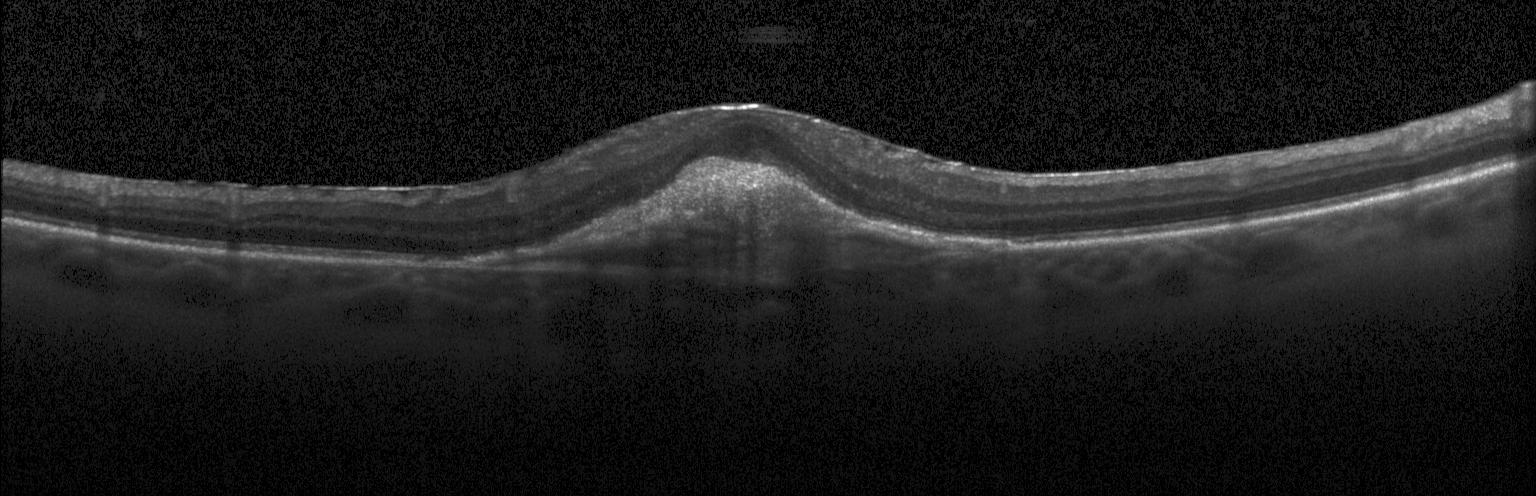
Acquired on a Heidelberg Spectralis · macular scan · OCT line scan.
Finding: a choroidal neovascular membrane.